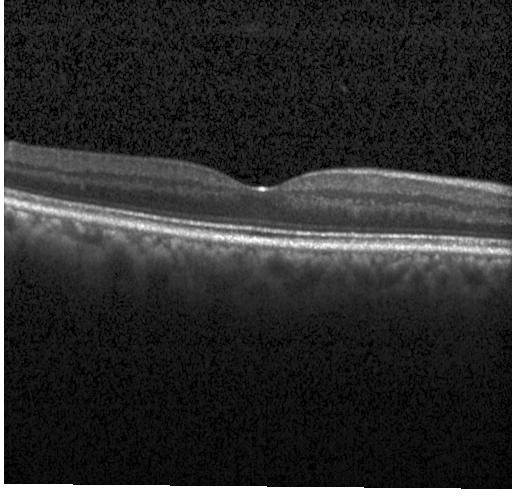

Macular OCT: no evidence of choroidal neovascularization, diabetic macular edema, or drusen.